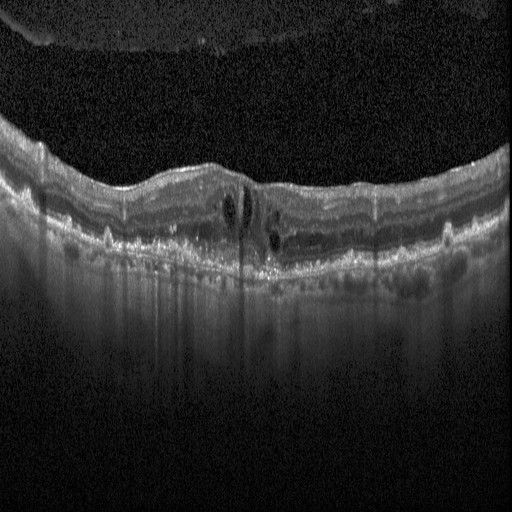
The scan shows DME.